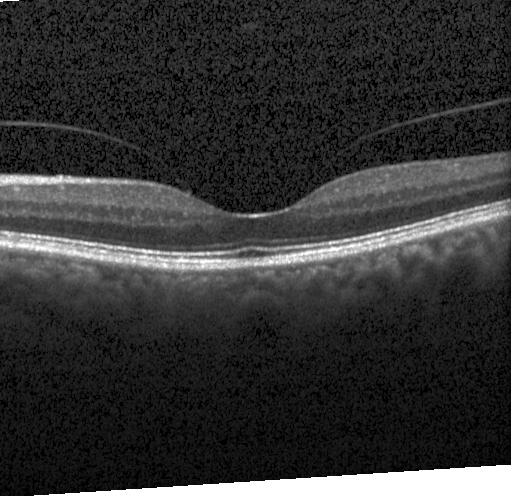

OCT line scan, through the macula, SD-OCT
Dx: no choroidal neovascularization, diabetic macular edema, or drusen.